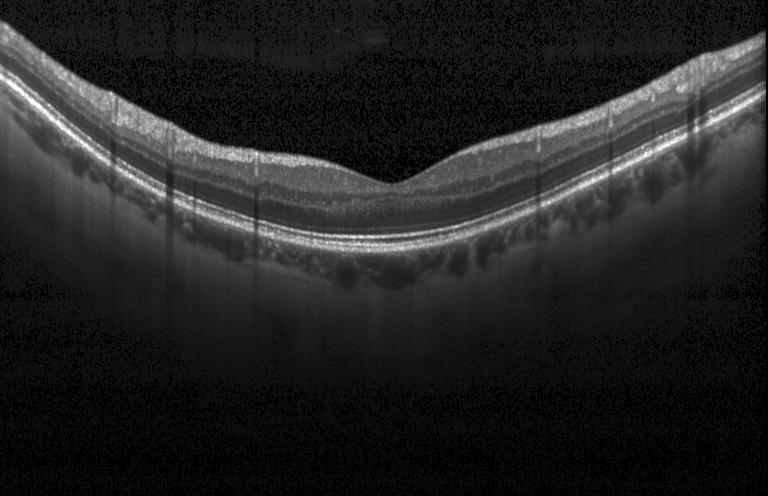
Retinal OCT cross-section — Dx: neither CNV, DME, nor drusen.